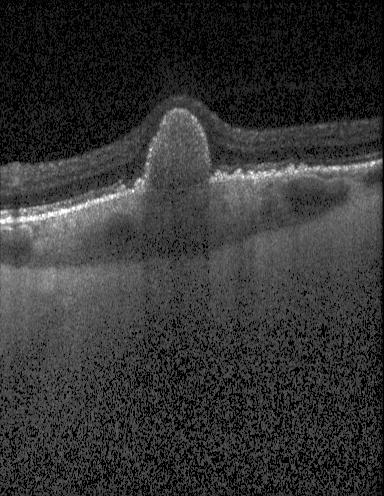 Optical coherence tomography scan · Heidelberg Spectralis · SD-OCT — Impression: a choroidal neovascular membrane.